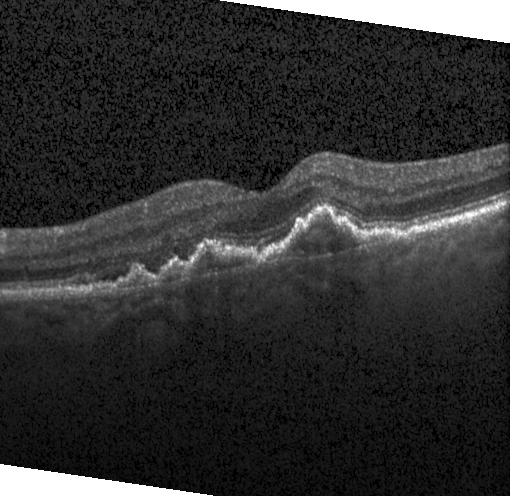

Optical coherence tomography B-scan. Assessment: choroidal neovascularization.